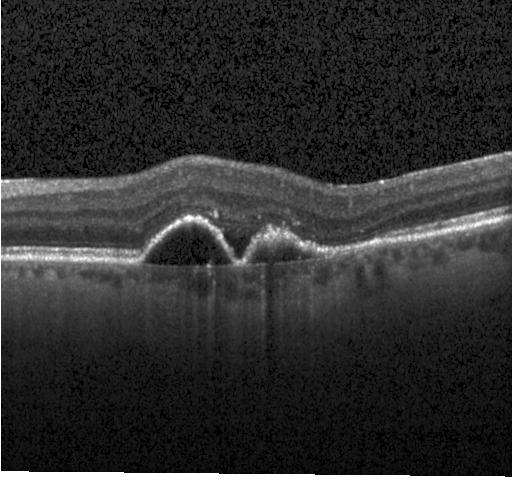

Spectral-domain optical coherence tomography; instrument: Heidelberg Spectralis; horizontal scan through the fovea; optical coherence tomography B-scan. Impression: a choroidal neovascular membrane.